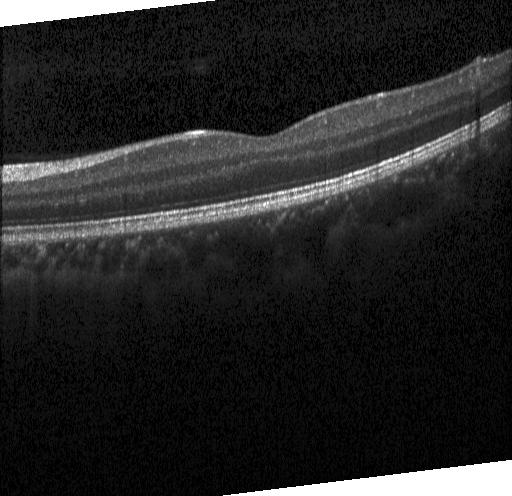
Retinal OCT B-scan. SD-OCT. Instrument: Heidelberg Spectralis. Fovea-centered. Finding: no evidence of CNV, DME, or drusen.